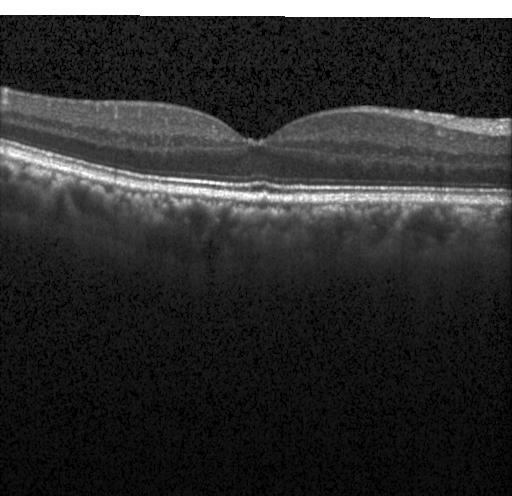

Diagnosis: multiple drusen.